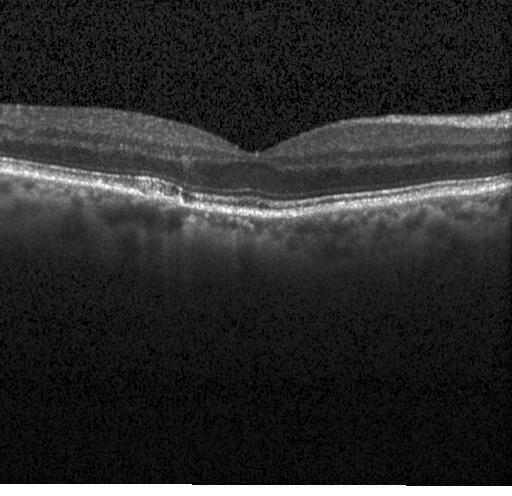

OCT line scan. Finding: drusen.